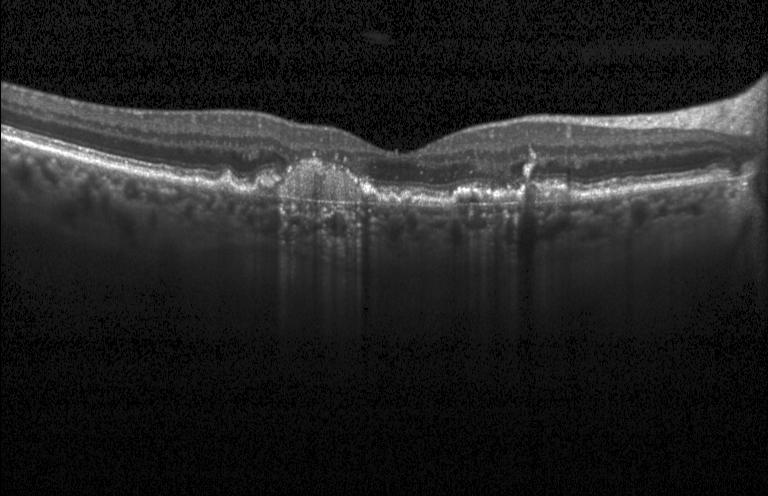

Optical coherence tomography scan; SD-OCT; acquired on a Heidelberg Spectralis; horizontal scan through the fovea.
The scan shows a choroidal neovascular membrane.